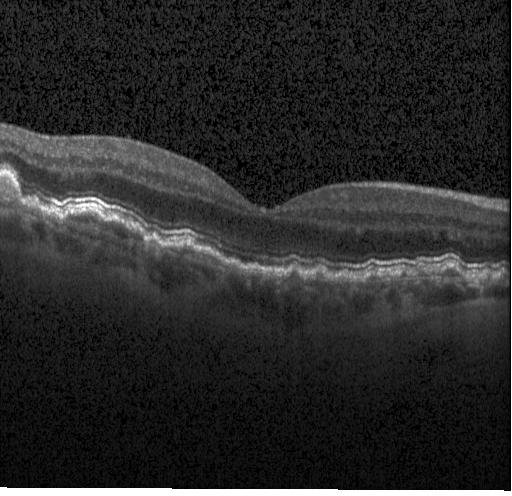

Impression: drusen.